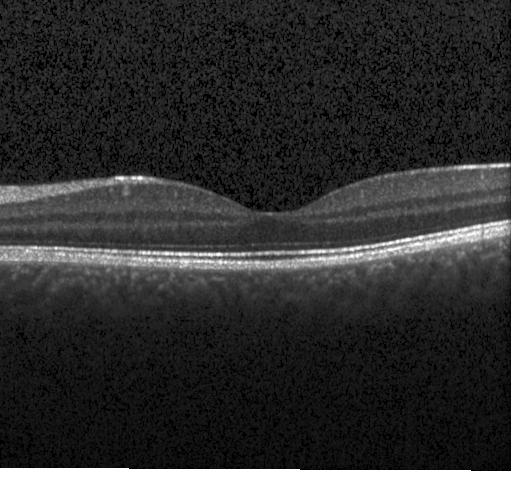

Instrument: Heidelberg Spectralis. Optical coherence tomography scan.
This B-scan demonstrates neither CNV, DME, nor drusen.